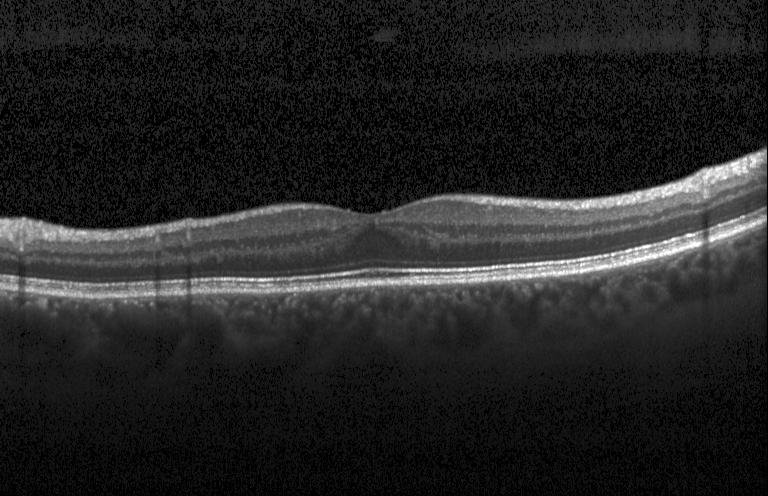
Finding: no choroidal neovascularization, no diabetic macular edema, and no drusen.